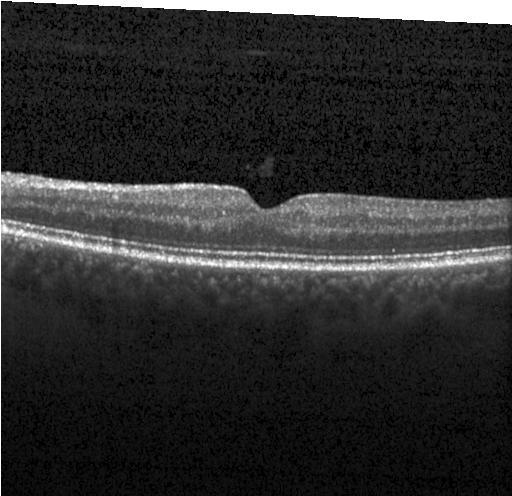

Retinal OCT cross-section; spectral-domain OCT
Impression: neither CNV, DME, nor drusen.